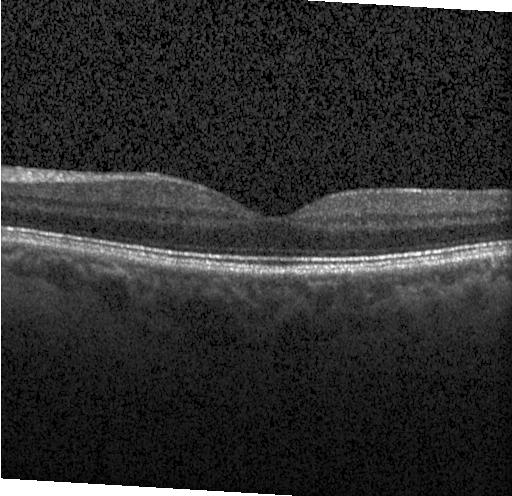 Dx: no evidence of choroidal neovascularization, diabetic macular edema, or drusen.